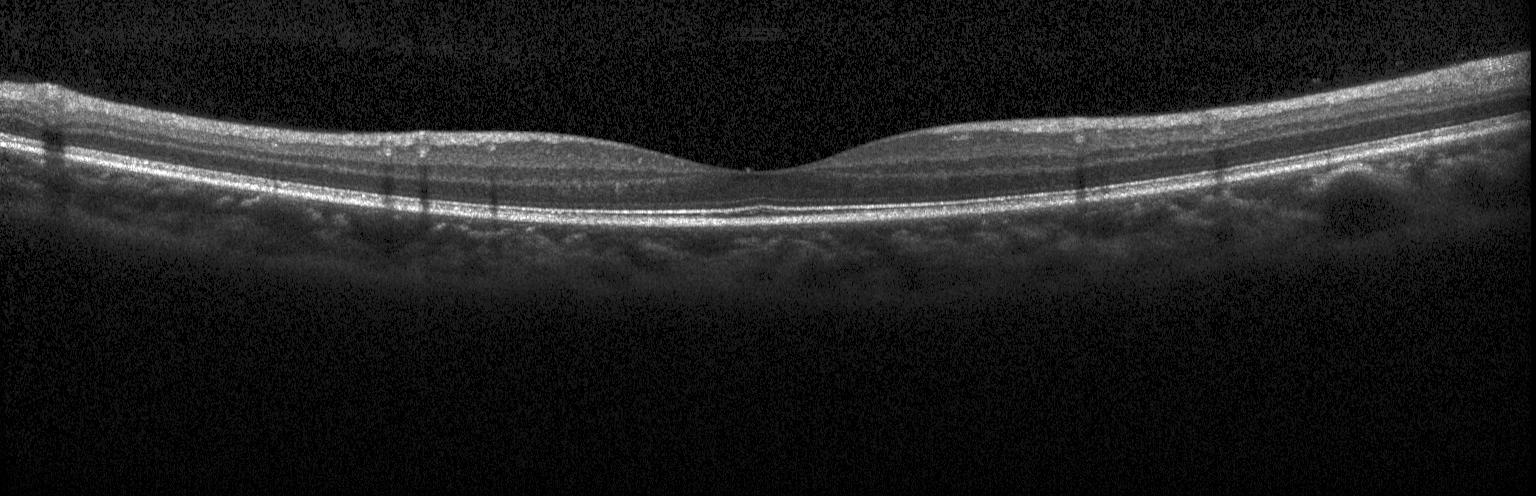

Retinal OCT cross-section — Finding: no evidence of choroidal neovascularization, diabetic macular edema, or drusen.